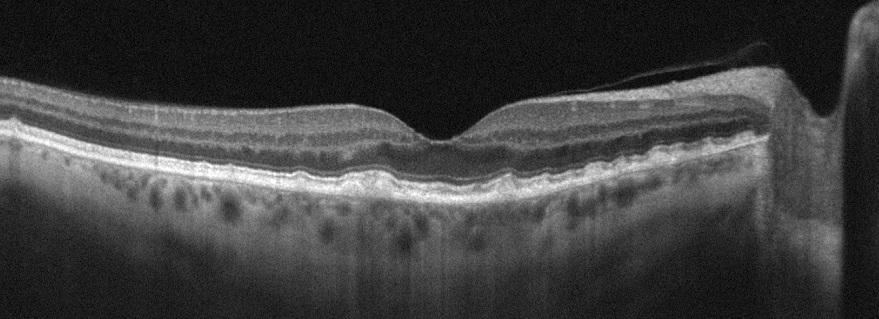 Through the macula, optical coherence tomography B-scan, acquired on an Optovue Avanti RTVue XR.
Diagnosis: AMD.